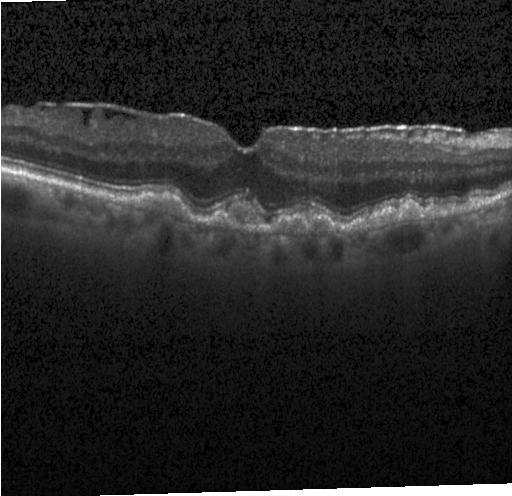
Retinal OCT B-scan.
Diagnosis: multiple drusen.